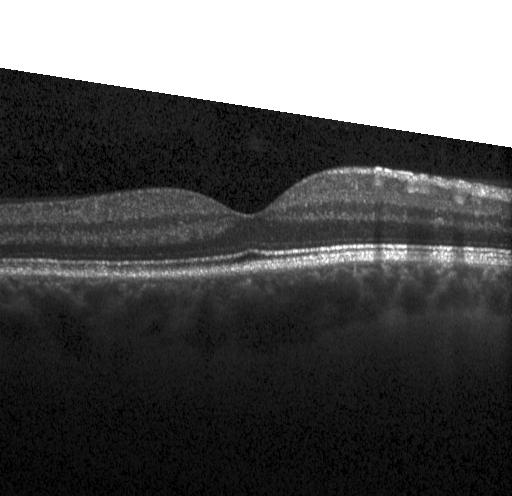

Macular scan · retinal OCT B-scan · SD-OCT · instrument: Heidelberg Spectralis. Diagnosis: no choroidal neovascularization, no diabetic macular edema, and no drusen.